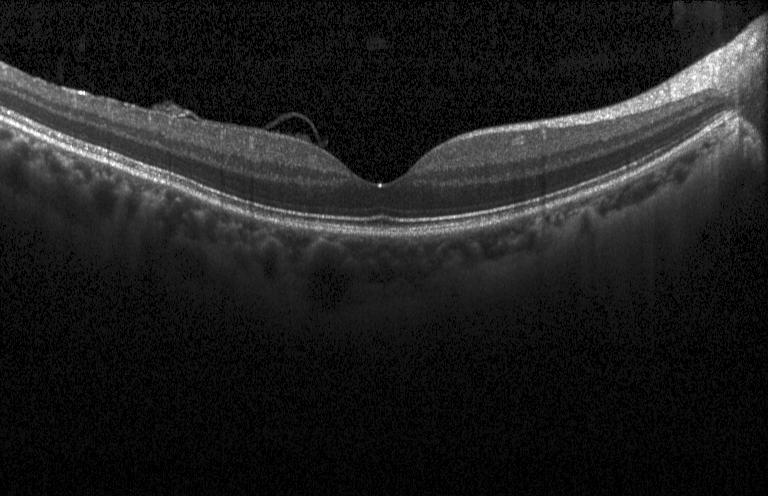
Optical coherence tomography B-scan.
Finding: no CNV, no DME, and no drusen.